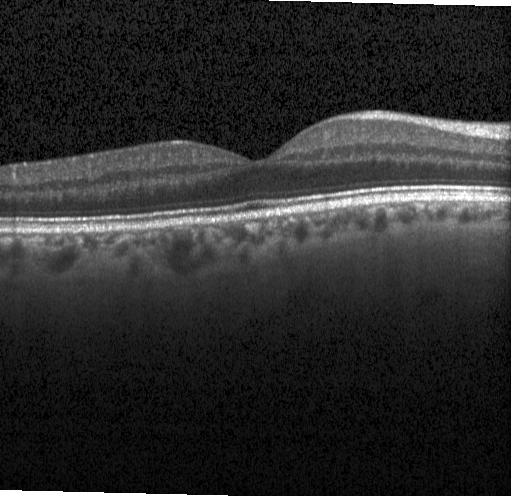
Macular scan. OCT B-scan
OCT finding: no choroidal neovascularization, diabetic macular edema, or drusen.